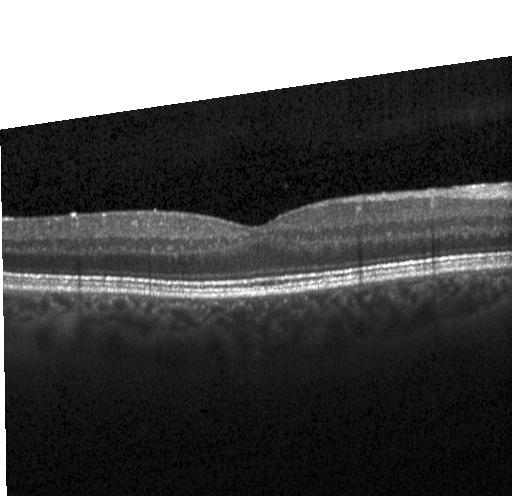

SD-OCT, optical coherence tomography B-scan. Assessment: no CNV, no DME, and no drusen.